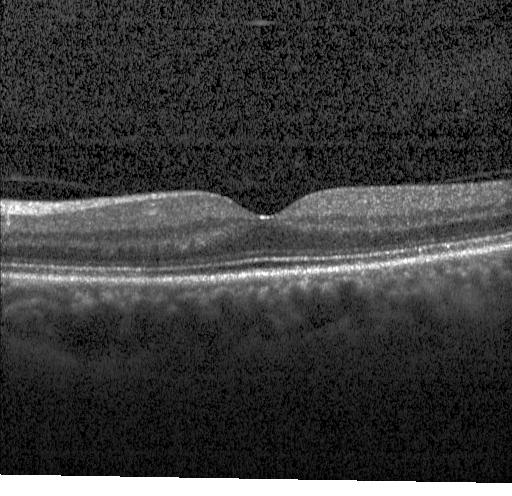

OCT B-scan showing no CNV, DME, or drusen.